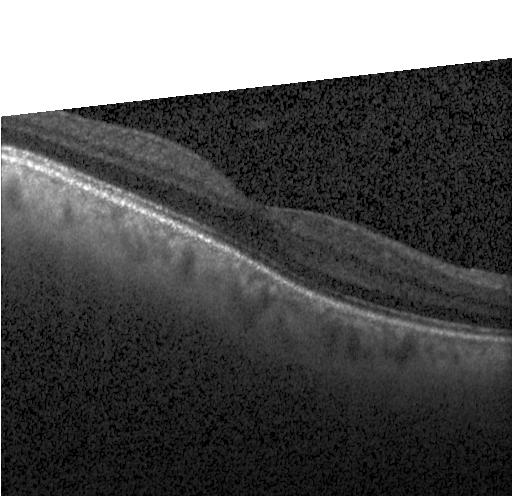 OCT finding: no choroidal neovascularization, no diabetic macular edema, and no drusen.